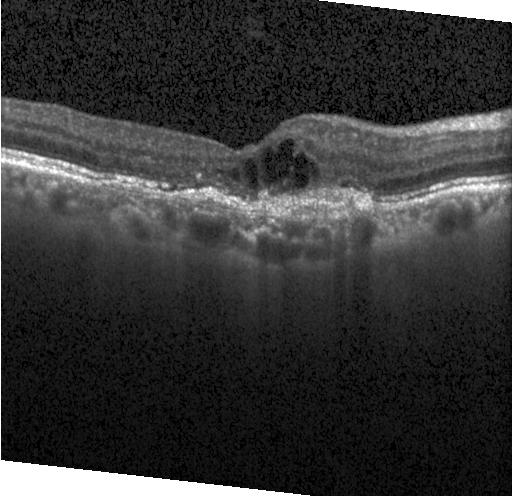
Retinal OCT B-scan, Heidelberg Spectralis OCT system, SD-OCT, centered on the fovea.
Diagnosis: a choroidal neovascular membrane.